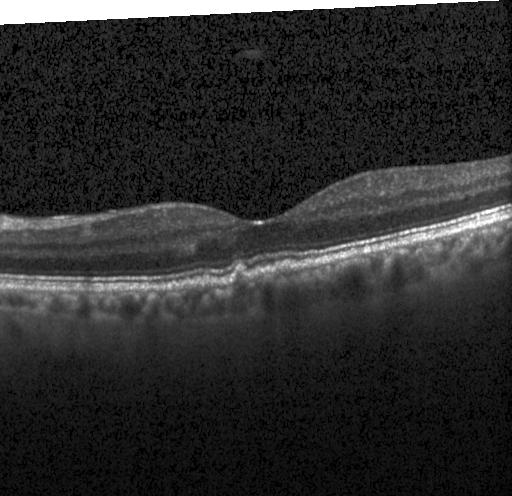 Optical coherence tomography B-scan
Diagnosis: drusen.